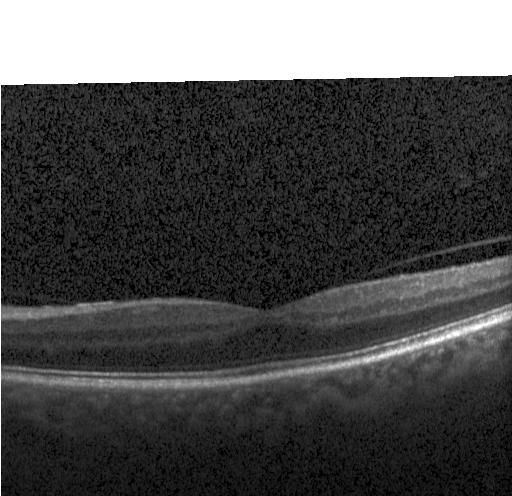
Retinal OCT cross-section. The scan shows no choroidal neovascularization, diabetic macular edema, or drusen.